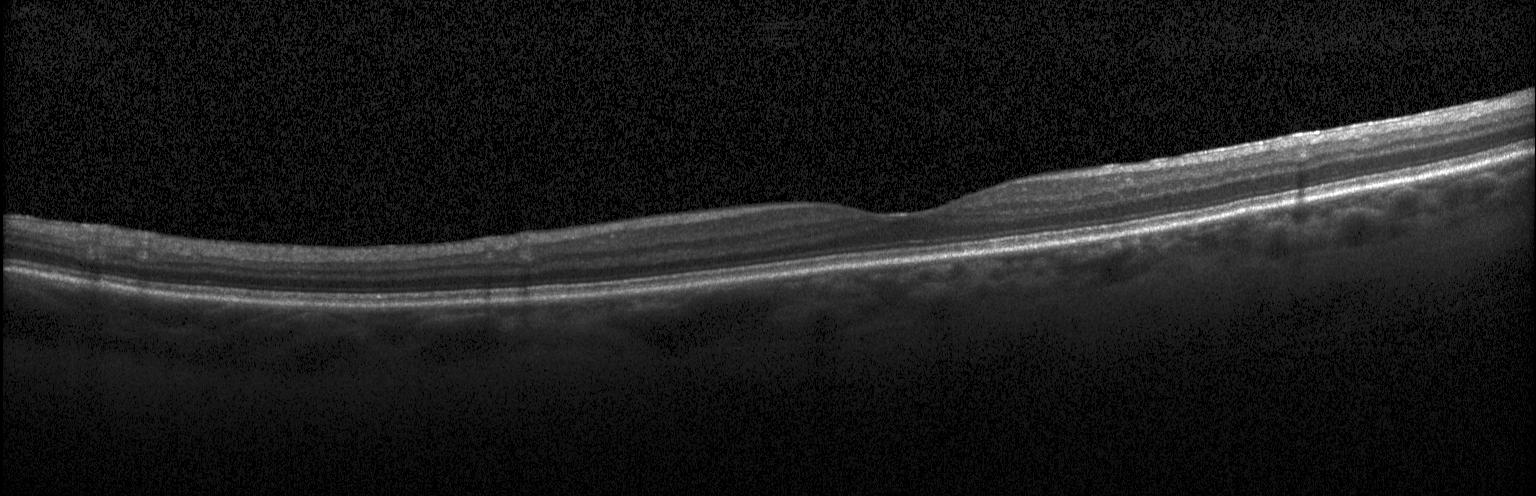 Spectral-domain optical coherence tomography · retinal OCT B-scan
Dx: no choroidal neovascularization, no diabetic macular edema, and no drusen.